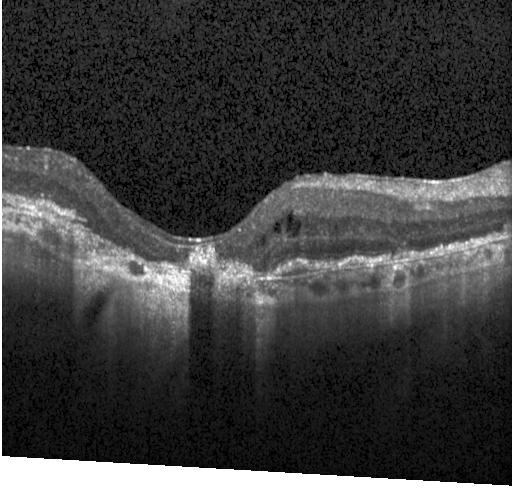
Heidelberg Spectralis OCT system. Horizontal scan through the fovea. Retinal OCT cross-section
The scan shows a choroidal neovascular membrane.